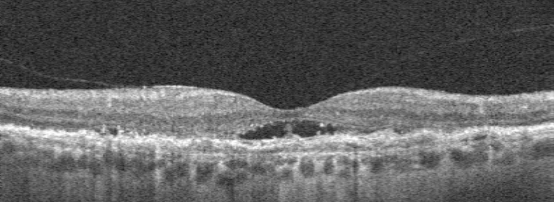 Optical coherence tomography B-scan; macular scan. Impression: age-related macular degeneration (AMD).